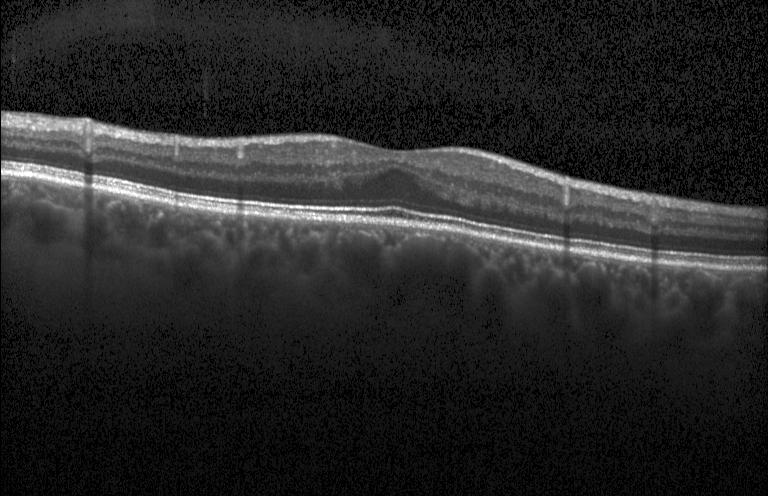 Horizontal scan through the fovea; spectral-domain optical coherence tomography; instrument: Heidelberg Spectralis; optical coherence tomography scan
The scan shows no choroidal neovascularization, diabetic macular edema, or drusen.